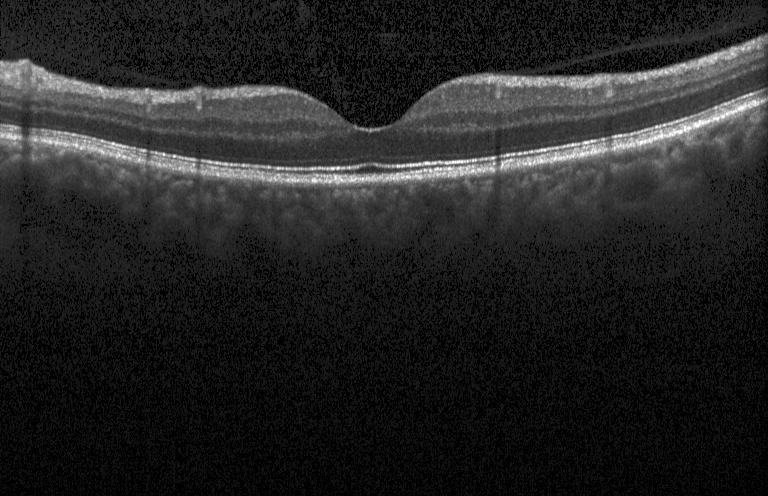

The scan shows no CNV, DME, or drusen.